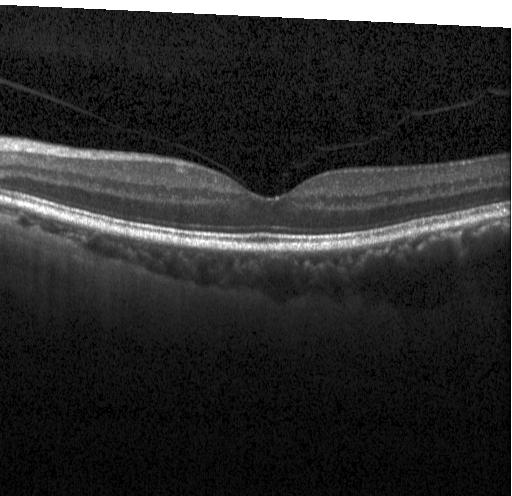

SD-OCT; optical coherence tomography B-scan; instrument: Heidelberg Spectralis; macular scan. Assessment: no CNV, DME, or drusen.